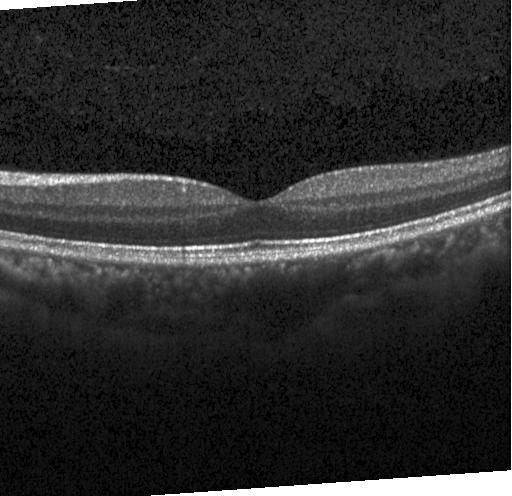

Retinal OCT cross-section. Finding: neither choroidal neovascularization, diabetic macular edema, nor drusen.